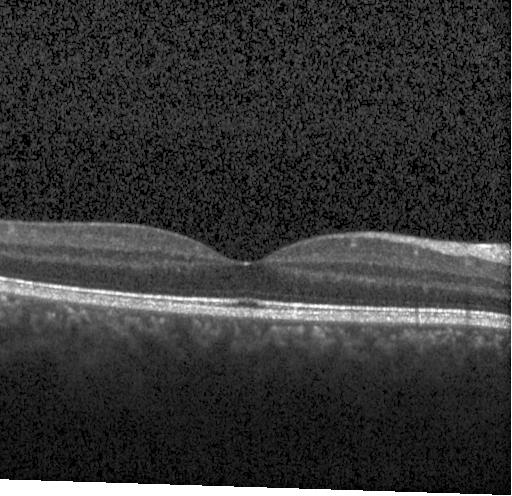

OCT finding: no CNV, DME, or drusen.